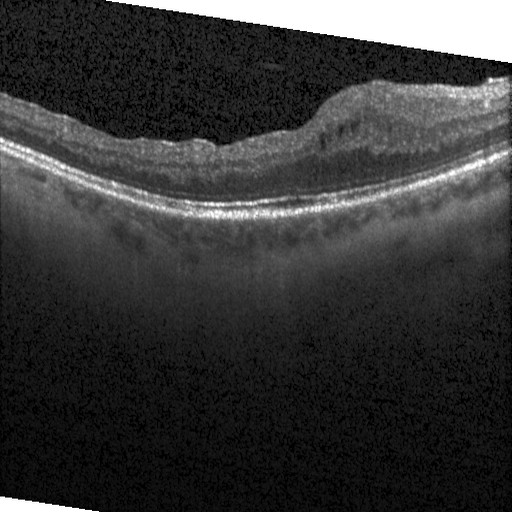
Retinal OCT B-scan · spectral-domain optical coherence tomography · horizontal scan through the fovea · Heidelberg Spectralis.
Macular OCT: diabetic macular edema (DME).